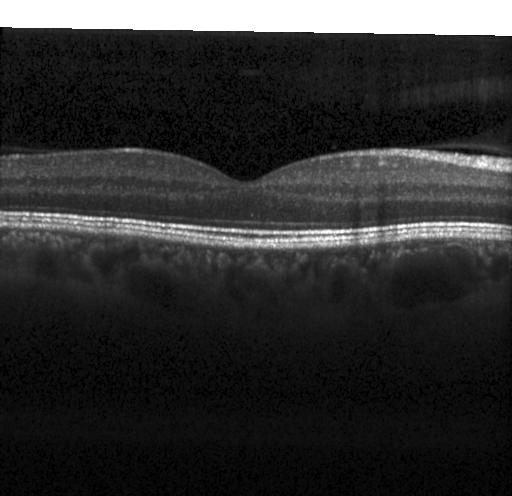
OCT line scan; fovea-centered; spectral-domain OCT; instrument: Heidelberg Spectralis
This B-scan demonstrates no choroidal neovascularization, diabetic macular edema, or drusen.